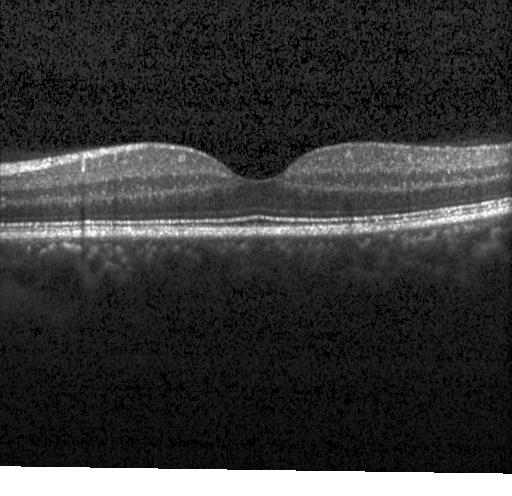

The scan shows neither choroidal neovascularization, diabetic macular edema, nor drusen.